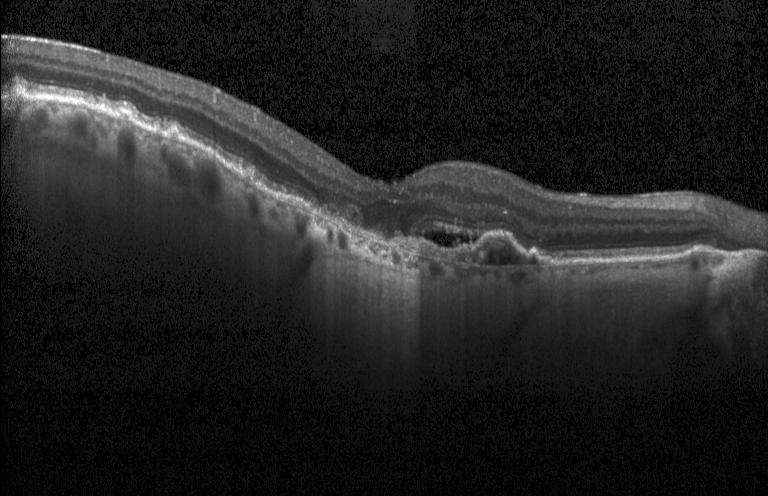

Retinal OCT cross-section showing a choroidal neovascular membrane.